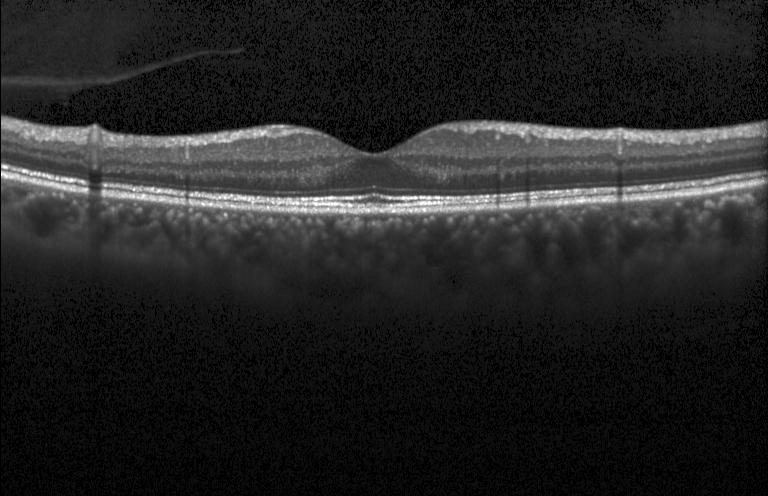

Spectral-domain OCT, retinal OCT B-scan. Assessment: no choroidal neovascularization, no diabetic macular edema, and no drusen.